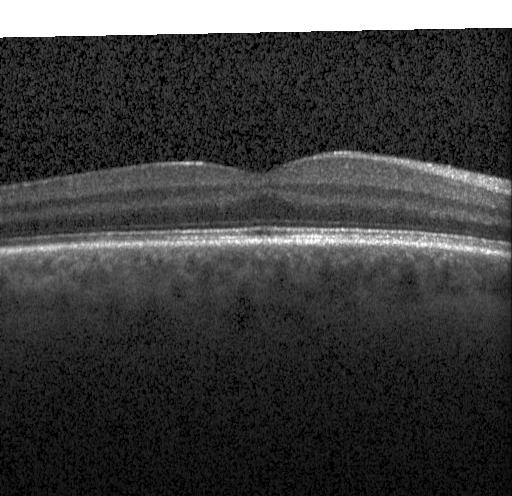

Impression: neither choroidal neovascularization, diabetic macular edema, nor drusen.